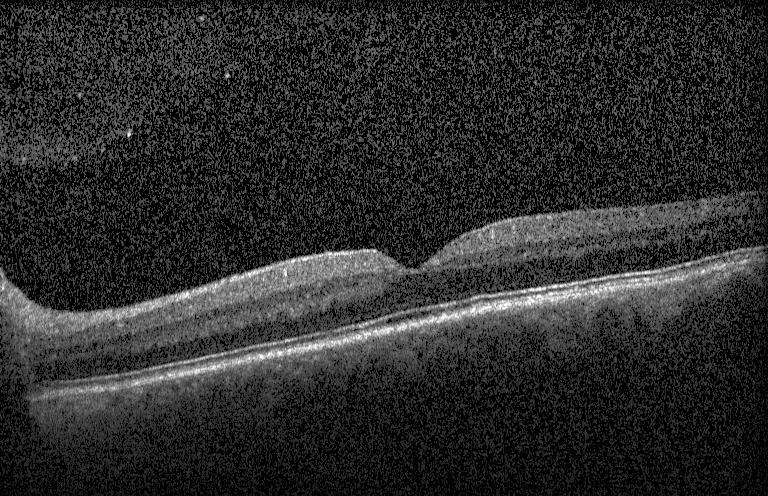 Optical coherence tomography B-scan, horizontal scan through the fovea, instrument: Heidelberg Spectralis
Impression: no choroidal neovascularization, no diabetic macular edema, and no drusen.